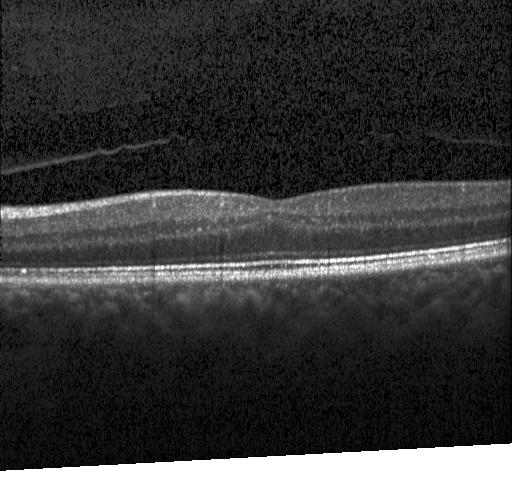 Retinal OCT cross-section showing no evidence of choroidal neovascularization, diabetic macular edema, or drusen.